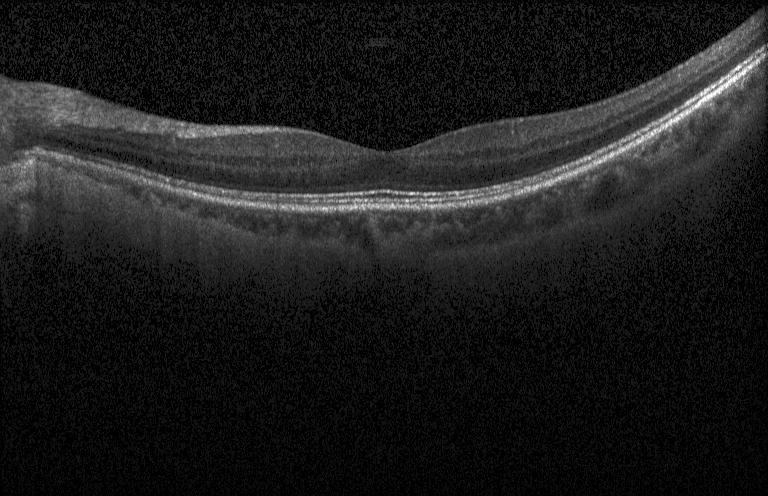
Macular OCT demonstrating no CNV, DME, or drusen.